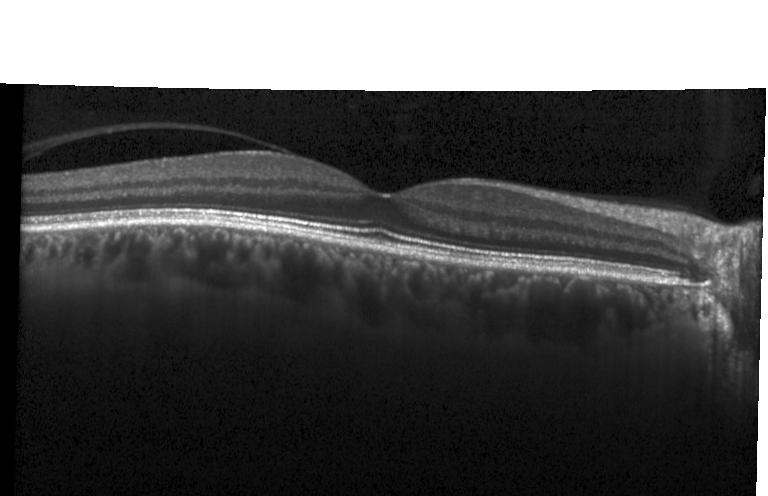 The scan shows neither choroidal neovascularization, diabetic macular edema, nor drusen.